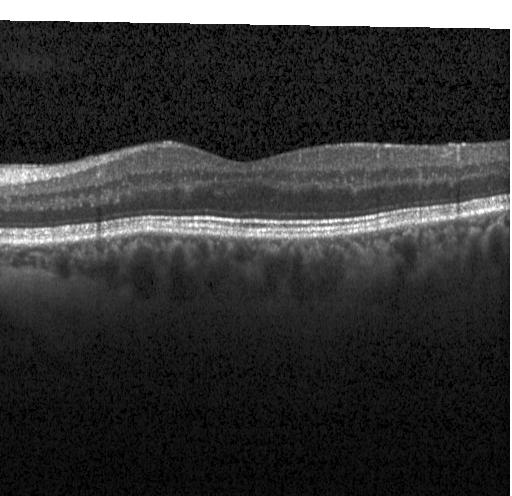

Impression: no evidence of choroidal neovascularization, diabetic macular edema, or drusen.